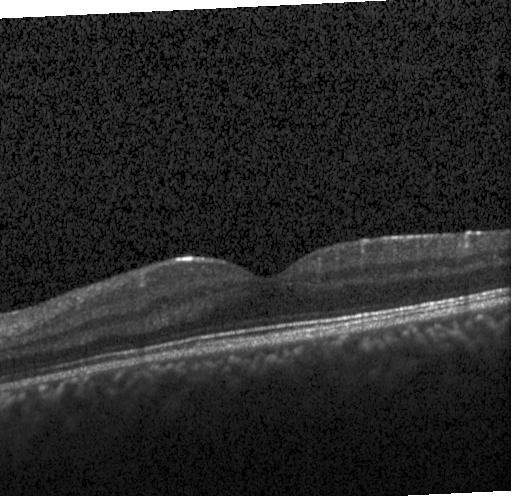
Fovea-centered; SD-OCT; retinal OCT B-scan — The scan shows no choroidal neovascularization, diabetic macular edema, or drusen.